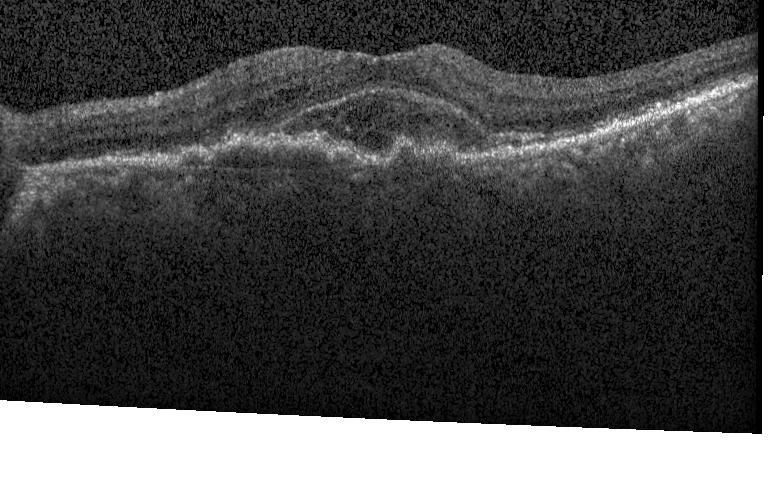 Optical coherence tomography scan. Diagnosis: CNV.